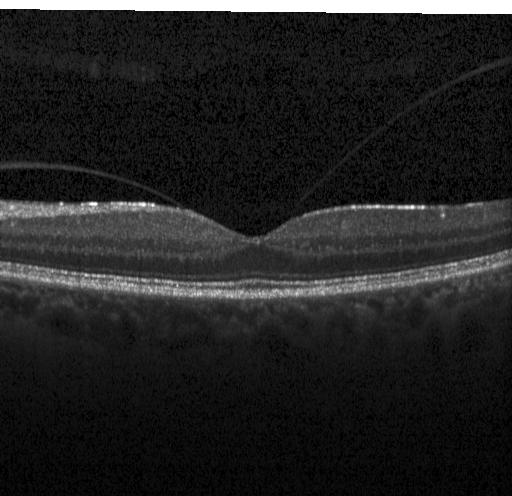 Spectral-domain OCT B-scan: neither choroidal neovascularization, diabetic macular edema, nor drusen.